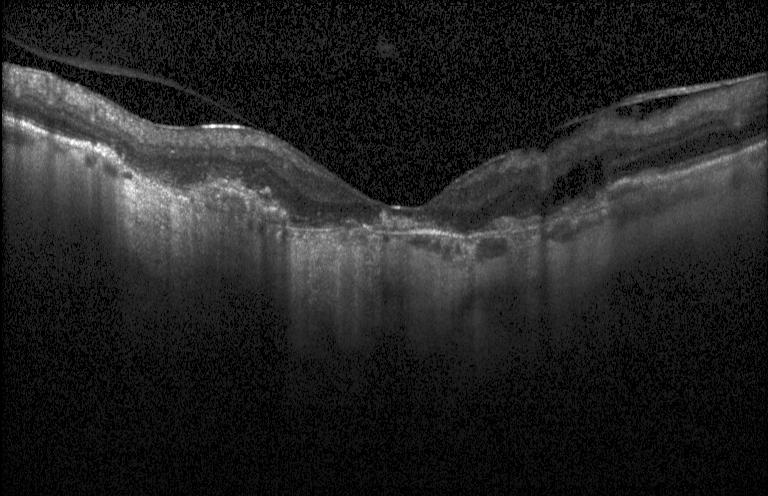
Diagnosis: a choroidal neovascular membrane.